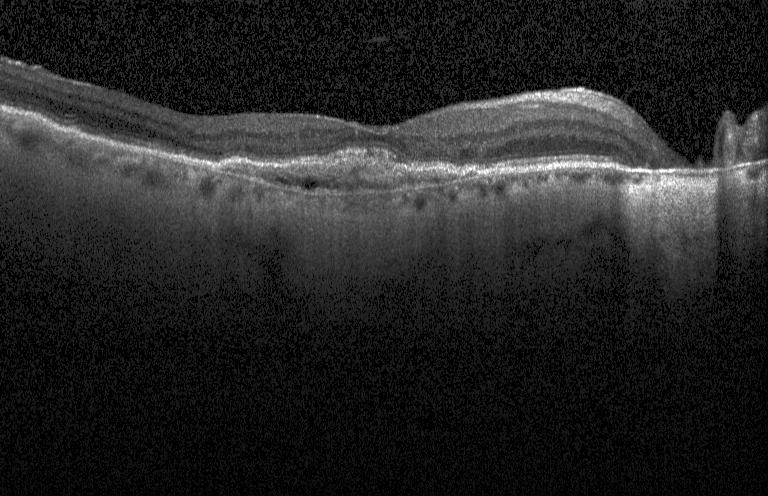 Optical coherence tomography B-scan — Impression: a choroidal neovascular membrane.